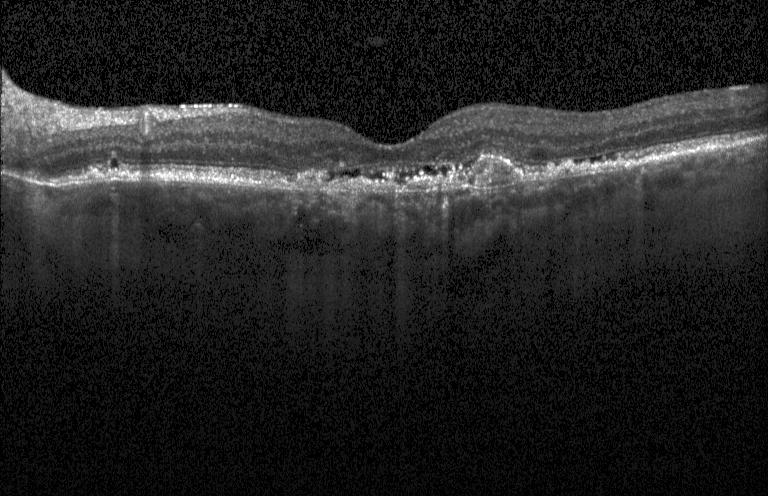 Spectral-domain OCT B-scan: CNV.